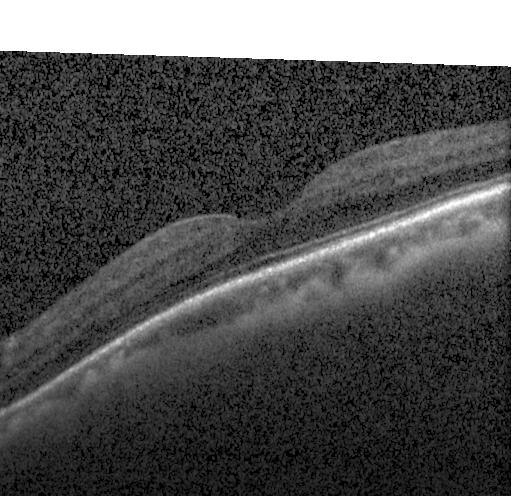
Acquired on a Heidelberg Spectralis; optical coherence tomography scan — Finding: no choroidal neovascularization, no diabetic macular edema, and no drusen.